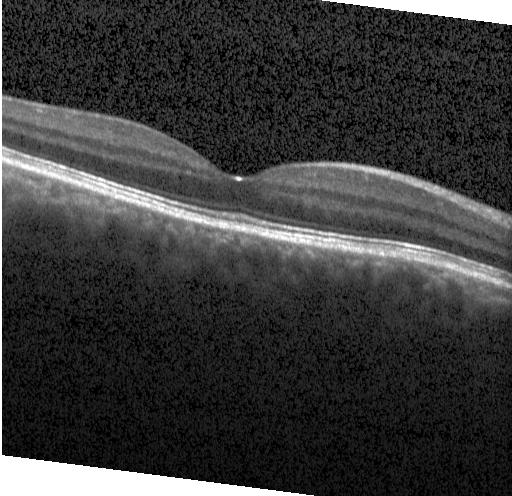 Heidelberg Spectralis OCT system, SD-OCT, retinal OCT cross-section, fovea-centered.
Diagnosis: no choroidal neovascularization, no diabetic macular edema, and no drusen.